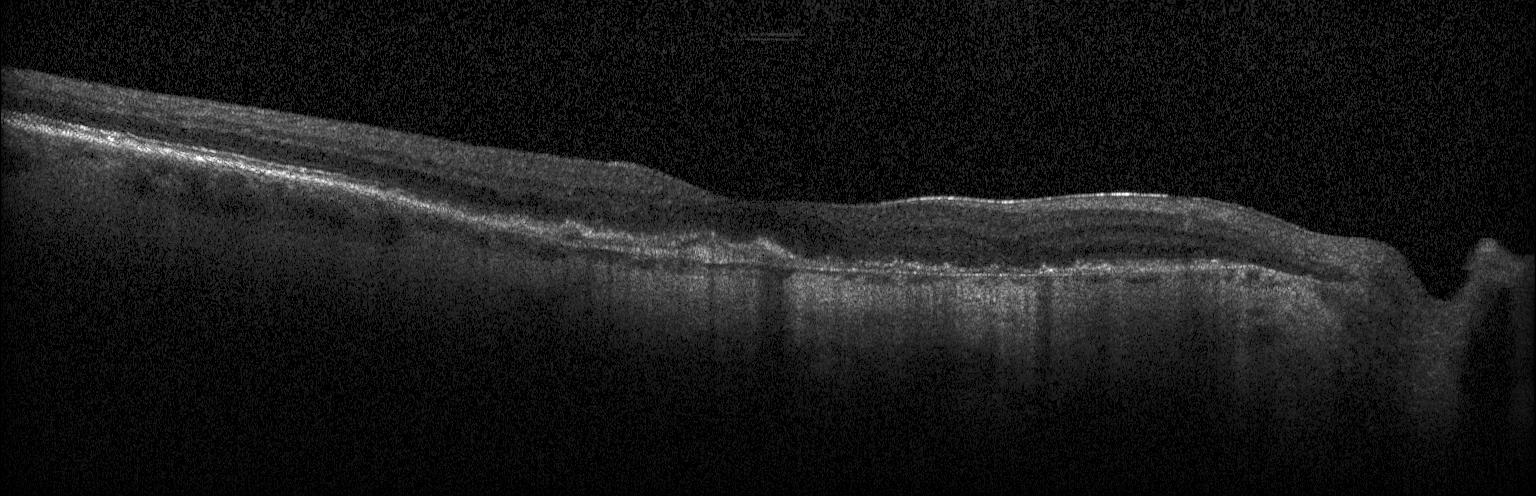 Macular OCT demonstrating CNV.